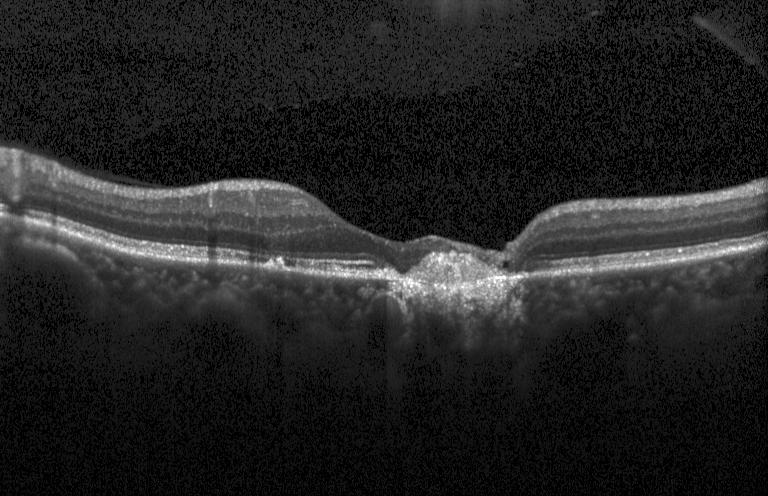 The scan shows choroidal neovascularization.